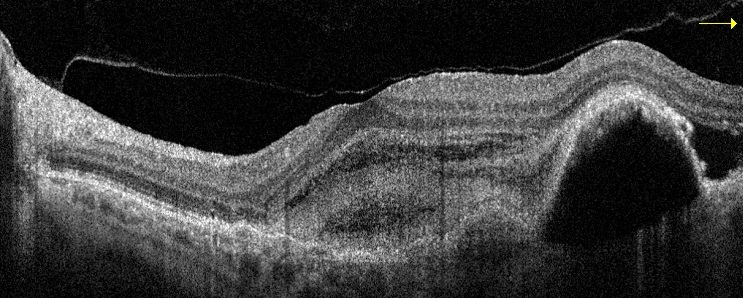

Retinal OCT cross-section showing AMD.